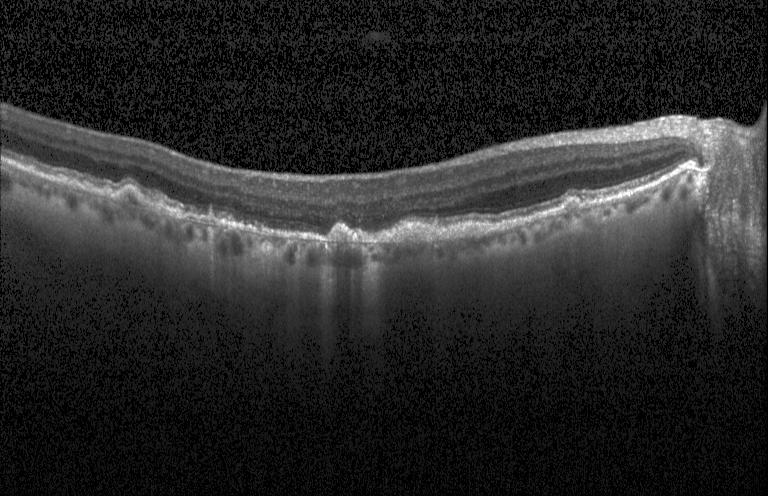

Impression: a choroidal neovascular membrane.